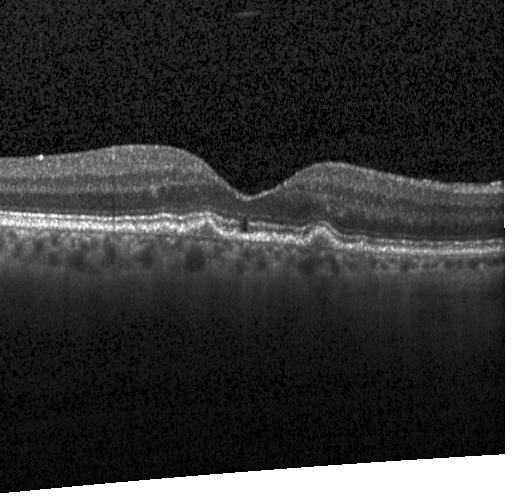
The scan shows multiple drusen.